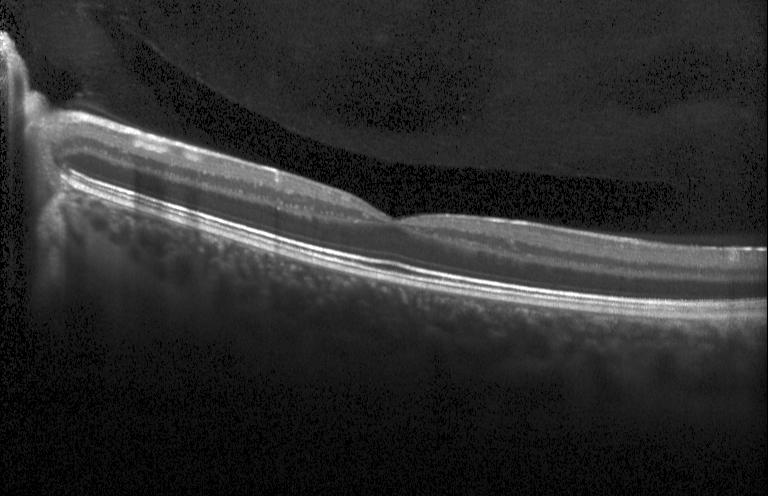
Diagnosis: no choroidal neovascularization, no diabetic macular edema, and no drusen.